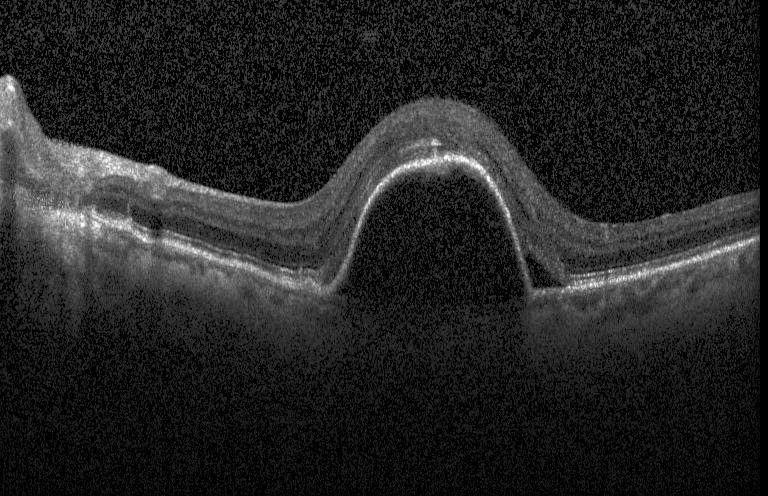

Optical coherence tomography scan, centered on the fovea, instrument: Heidelberg Spectralis, spectral-domain optical coherence tomography.
Finding: a choroidal neovascular membrane.